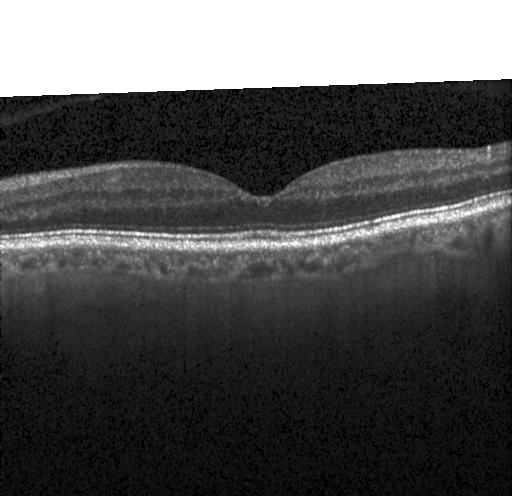 Finding: no choroidal neovascularization, no diabetic macular edema, and no drusen.